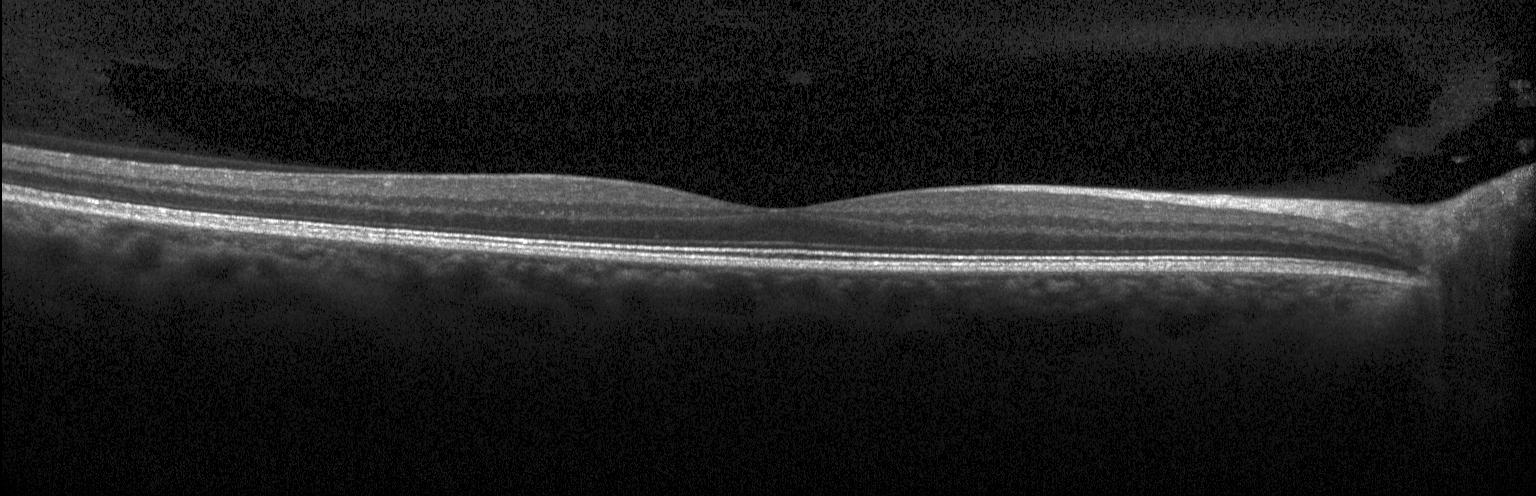
Horizontal scan through the fovea. OCT B-scan. Heidelberg Spectralis OCT system. Impression: no evidence of choroidal neovascularization, diabetic macular edema, or drusen.